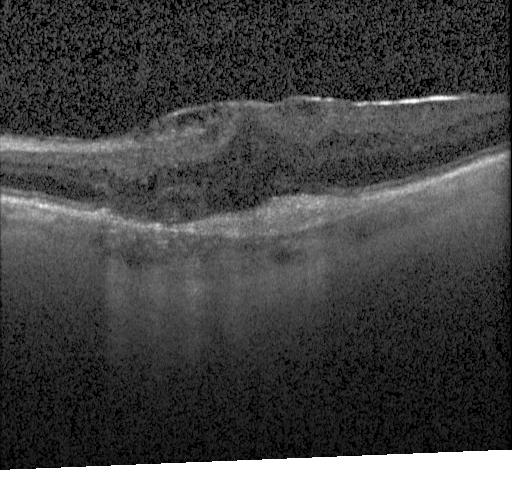 Macular scan. Spectral-domain optical coherence tomography. Optical coherence tomography scan. Heidelberg Spectralis
Finding: a choroidal neovascular membrane.